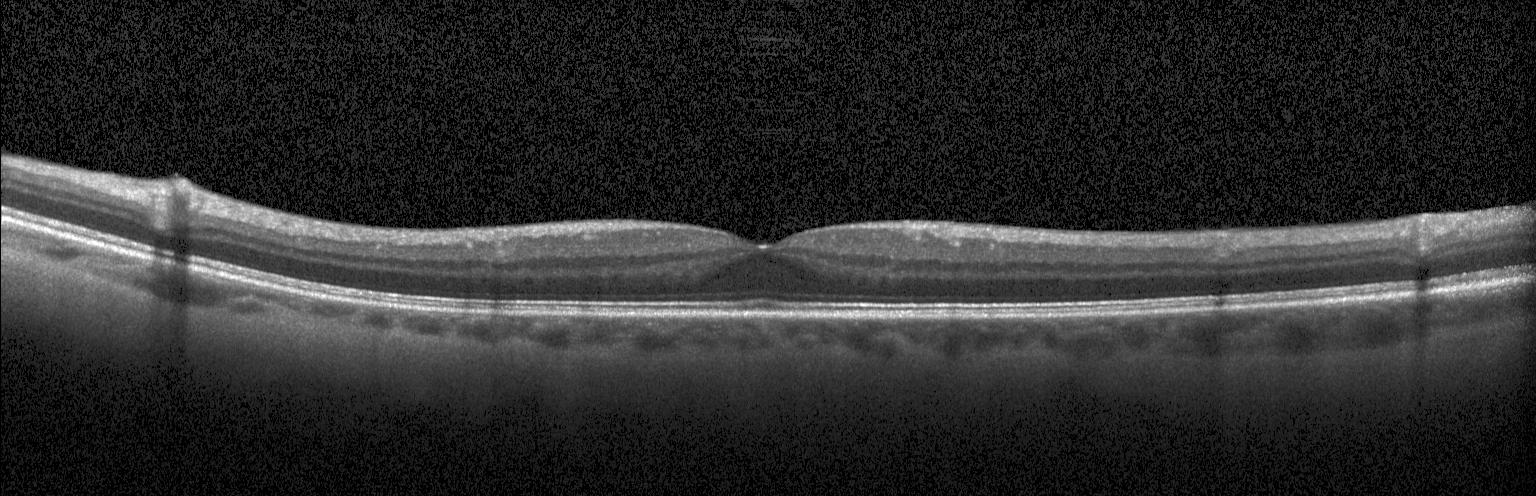

OCT B-scan showing no CNV, DME, or drusen.